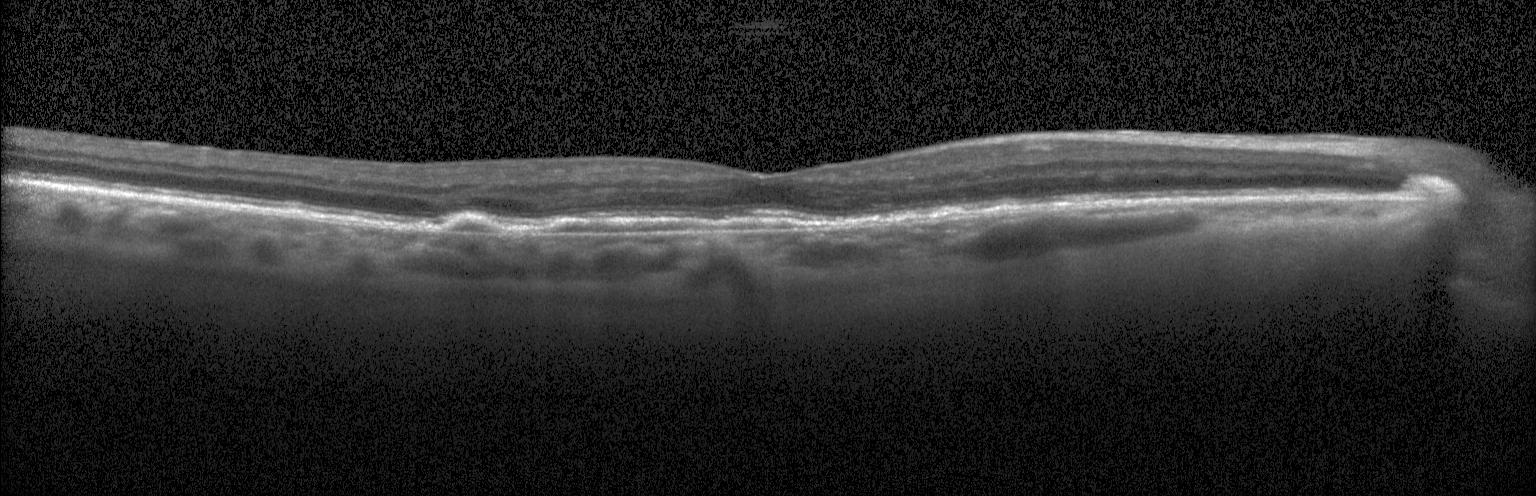
Optical coherence tomography B-scan, Heidelberg Spectralis OCT system. Impression: CNV.